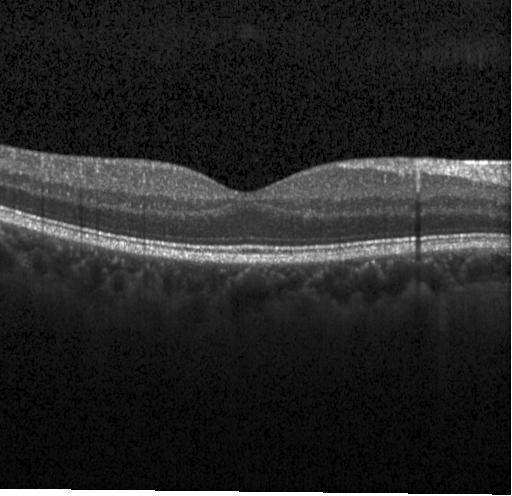

OCT B-scan. Finding: no CNV, DME, or drusen.